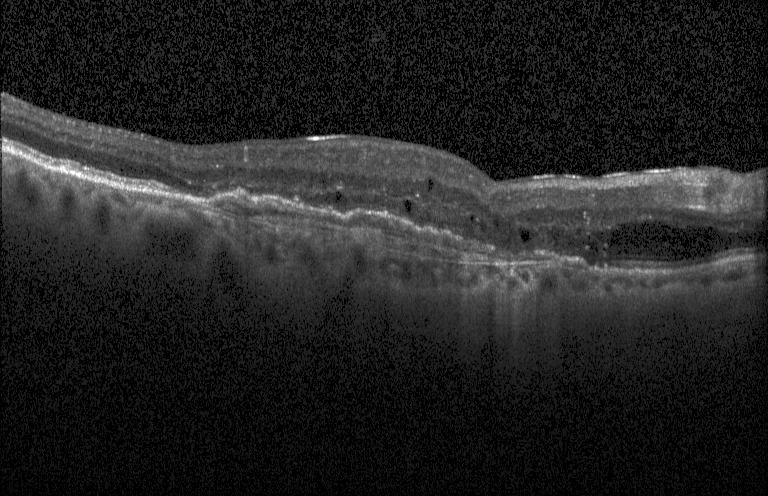

Acquired on a Heidelberg Spectralis. Optical coherence tomography scan. Macular scan.
Macular OCT: choroidal neovascularization.